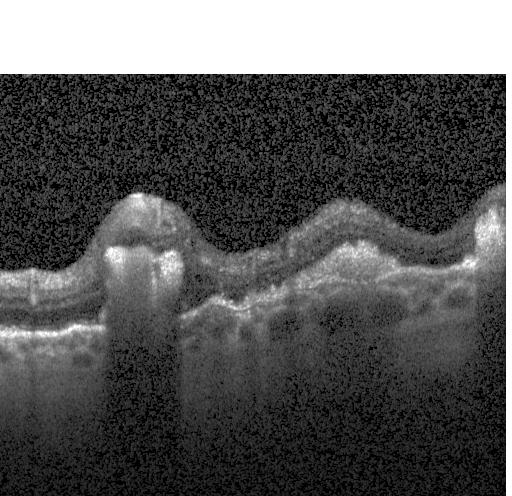
Retinal OCT cross-section. Finding: CNV.